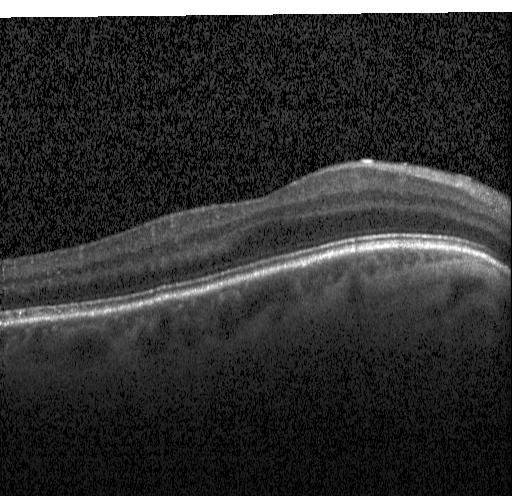
Spectral-domain optical coherence tomography, instrument: Heidelberg Spectralis, OCT B-scan
This B-scan demonstrates no evidence of choroidal neovascularization, diabetic macular edema, or drusen.